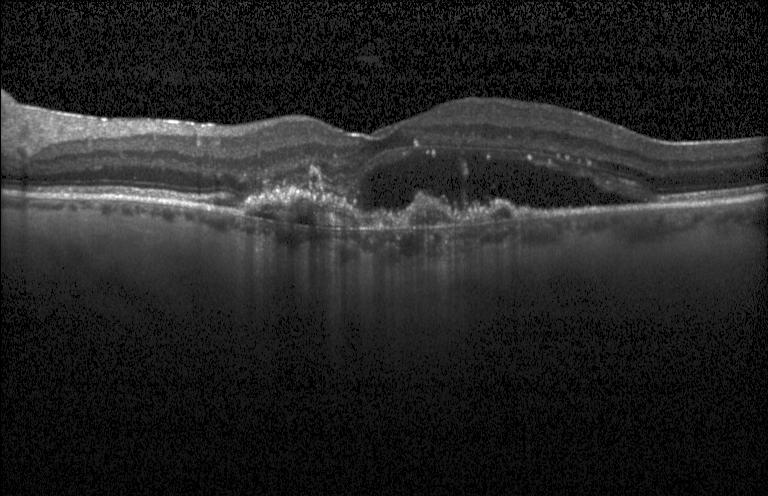 OCT B-scan · instrument: Heidelberg Spectralis · spectral-domain OCT.
Diagnosis: CNV.